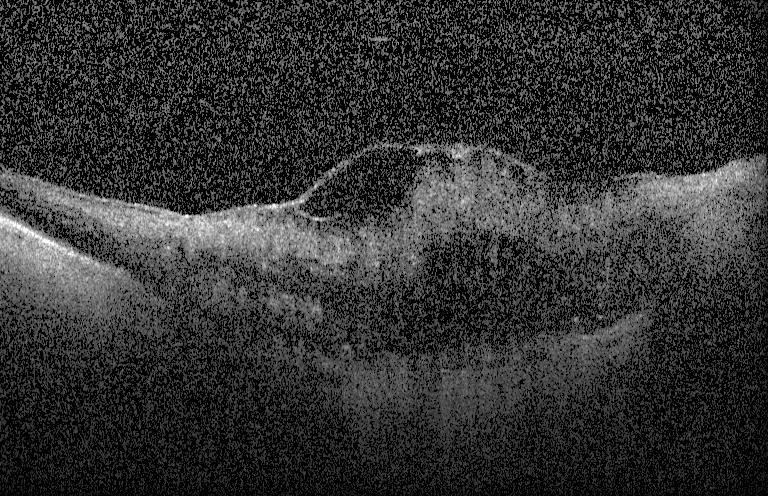 Optical coherence tomography scan.
The scan shows choroidal neovascularization.